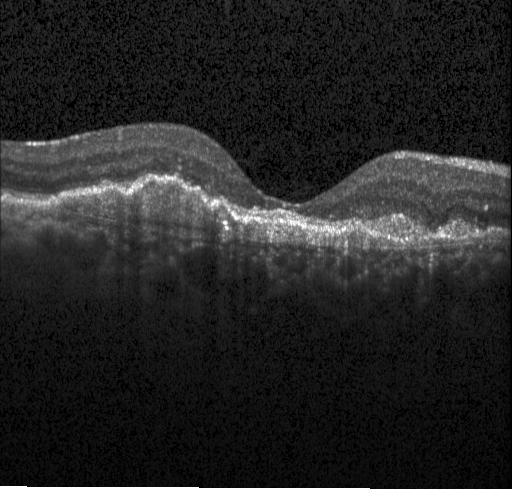

Dx: a choroidal neovascular membrane.